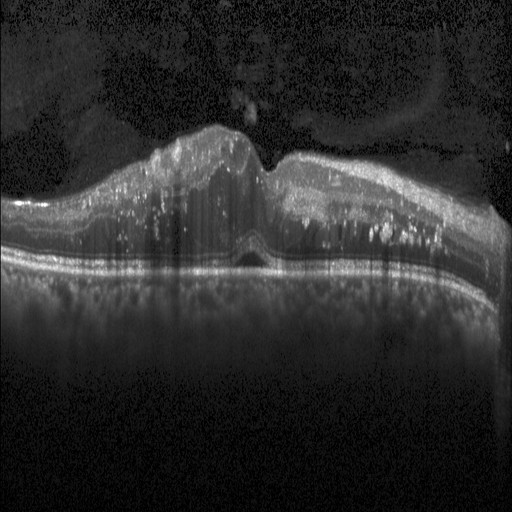
Finding: diabetic macular edema.